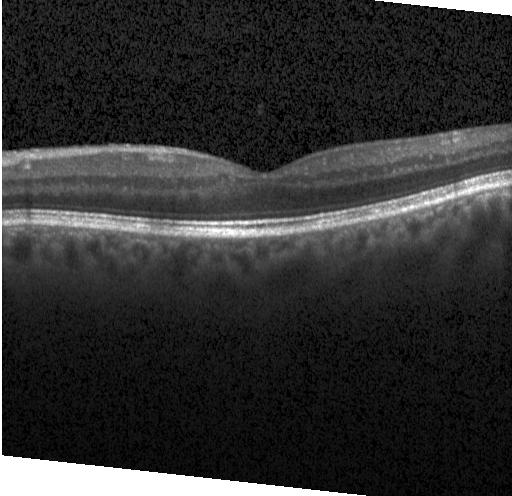

Diagnosis: no choroidal neovascularization, no diabetic macular edema, and no drusen.